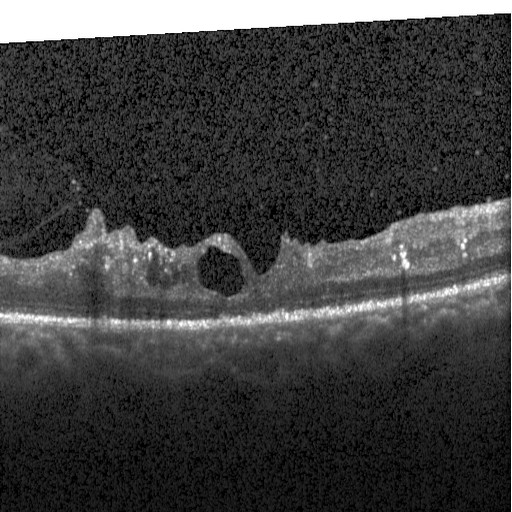
Impression: diabetic macular edema (DME).